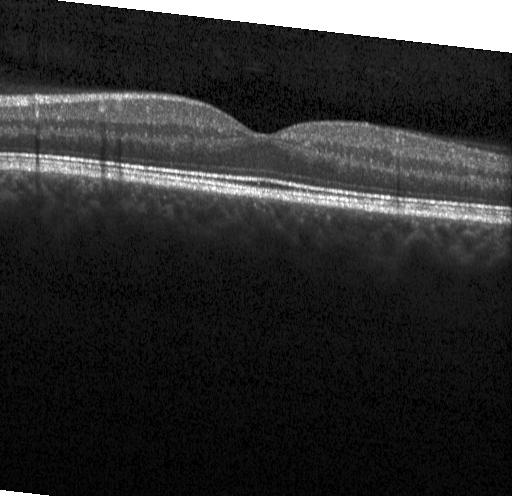 Through the macula; spectral-domain optical coherence tomography; optical coherence tomography scan; Heidelberg Spectralis OCT system — Impression: no choroidal neovascularization, no diabetic macular edema, and no drusen.